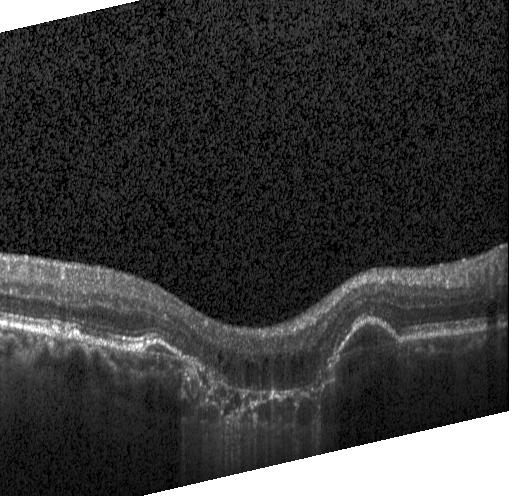
Finding: a choroidal neovascular membrane.